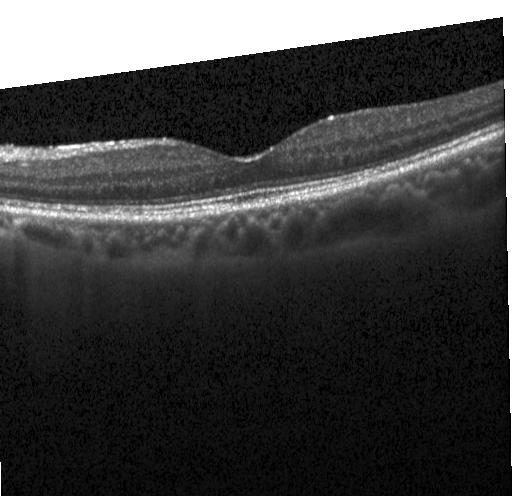

Diagnosis: no CNV, DME, or drusen.